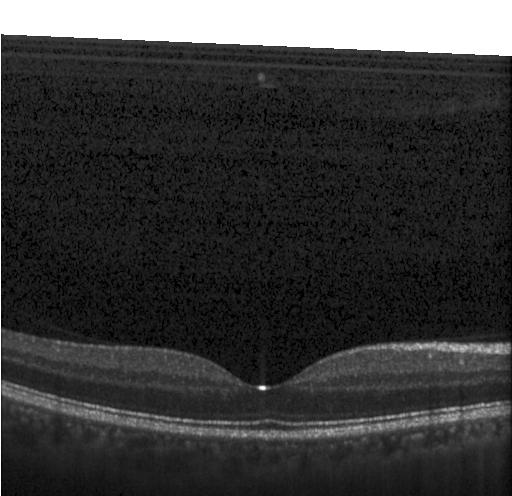
Assessment: no choroidal neovascularization, diabetic macular edema, or drusen.